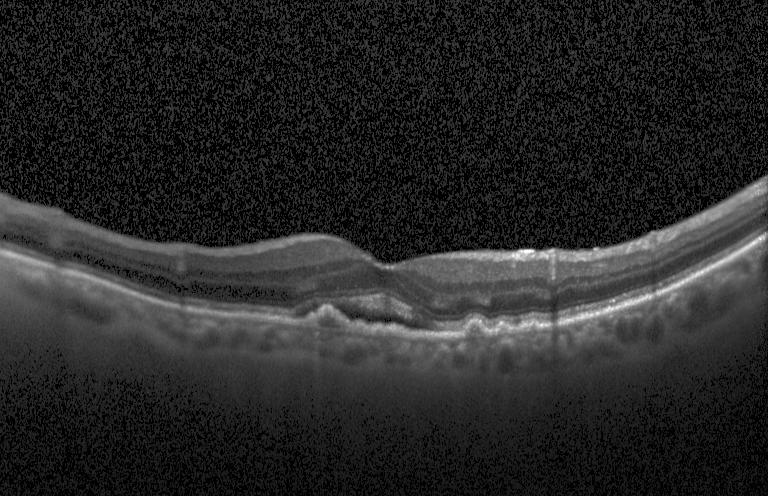

Finding: a choroidal neovascular membrane.